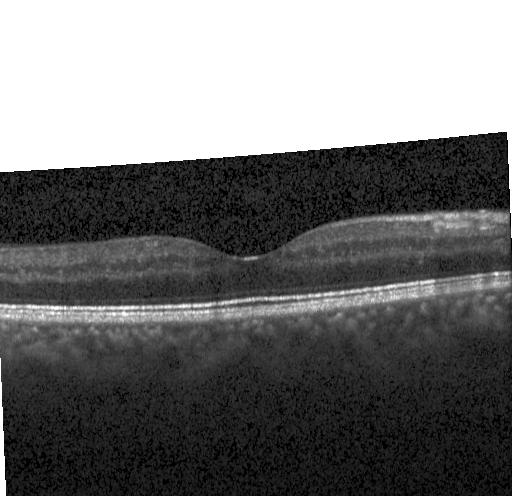

Dx: no CNV, DME, or drusen.